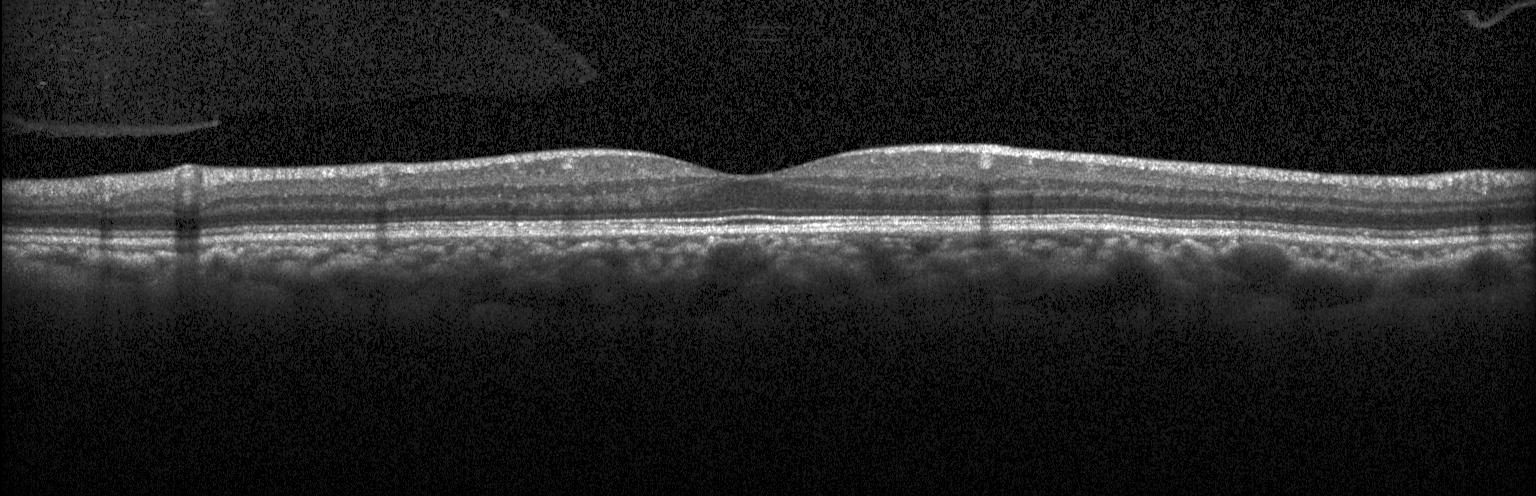 Through the macula. Spectral-domain optical coherence tomography. Optical coherence tomography scan. Heidelberg Spectralis.
Finding: neither CNV, DME, nor drusen.